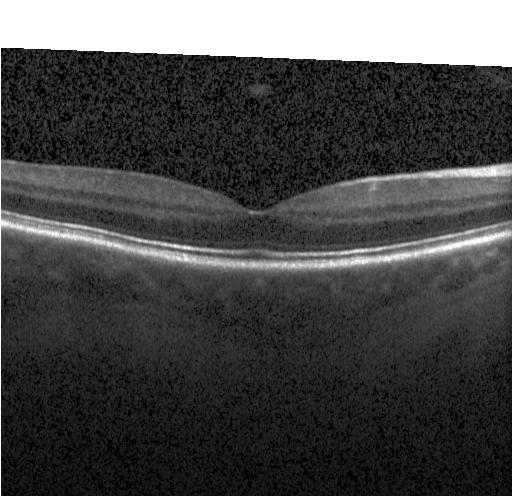
OCT B-scan
Finding: neither choroidal neovascularization, diabetic macular edema, nor drusen.